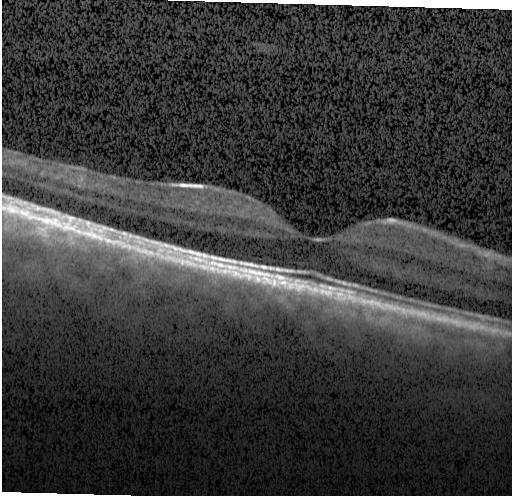 SD-OCT · instrument: Heidelberg Spectralis · optical coherence tomography scan — Dx: no evidence of CNV, DME, or drusen.